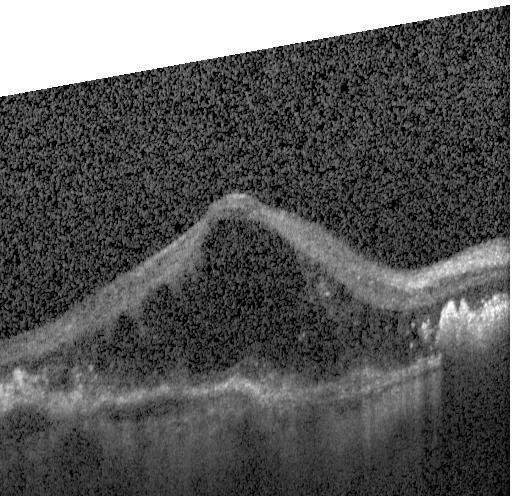

Optical coherence tomography B-scan; acquired on a Heidelberg Spectralis — Diagnosis: a choroidal neovascular membrane.